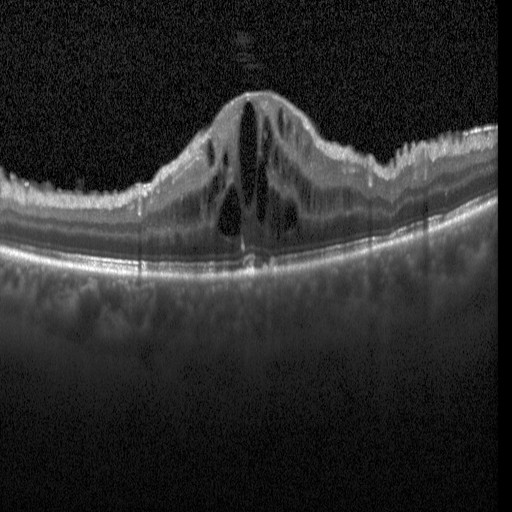
Heidelberg Spectralis OCT system; optical coherence tomography scan; fovea-centered. DME.